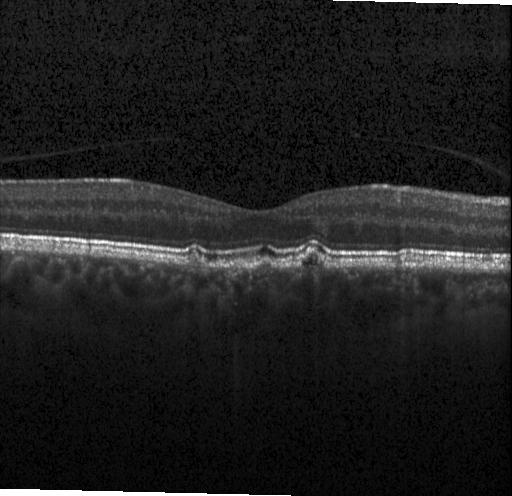
Retinal OCT cross-section · spectral-domain optical coherence tomography · macular scan. Dx: multiple drusen.